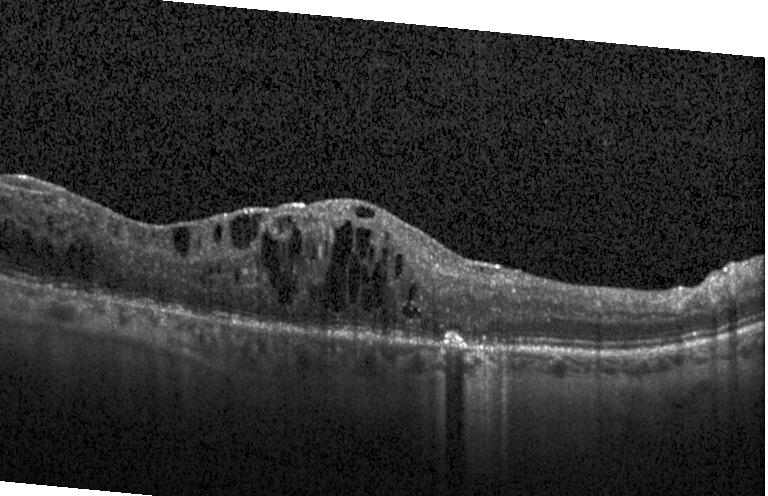
Finding: diabetic macular edema (DME).